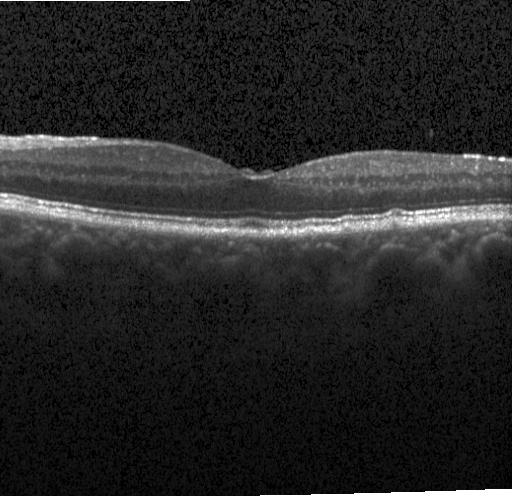

OCT line scan — Macular OCT: sub-RPE drusenoid deposits.